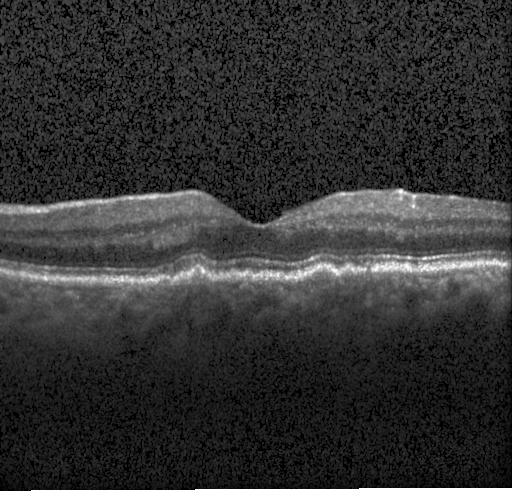
Acquired on a Heidelberg Spectralis; SD-OCT; macular scan; optical coherence tomography scan.
Diagnosis: multiple drusen.